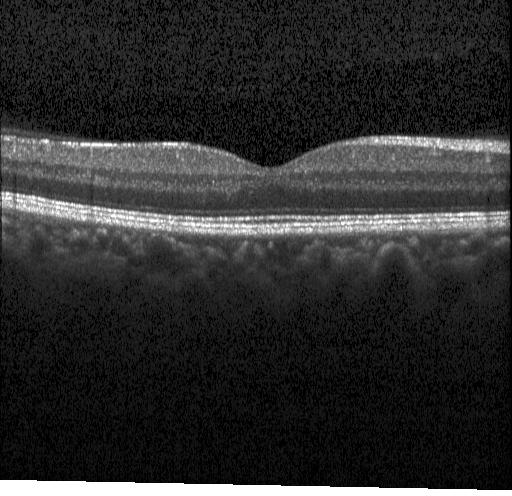

Optical coherence tomography B-scan, Heidelberg Spectralis — Dx: no CNV, no DME, and no drusen.